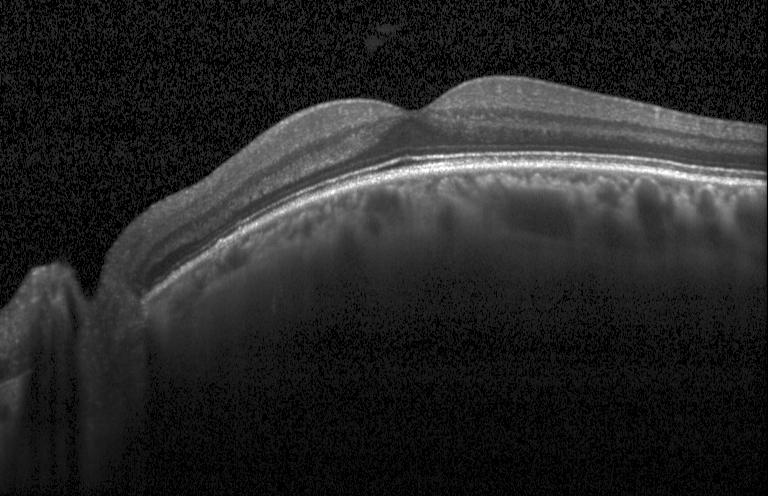
OCT B-scan showing no choroidal neovascularization, diabetic macular edema, or drusen.